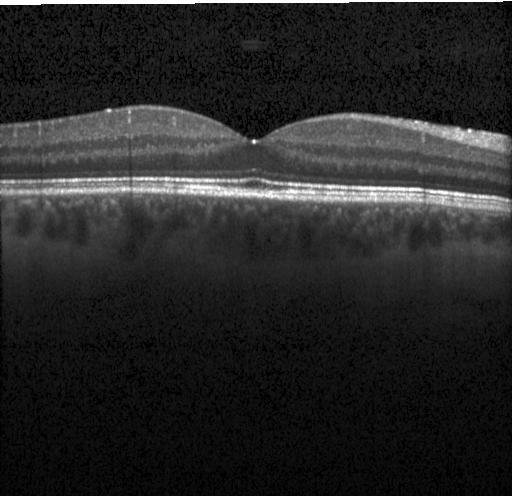 Impression: no evidence of choroidal neovascularization, diabetic macular edema, or drusen.